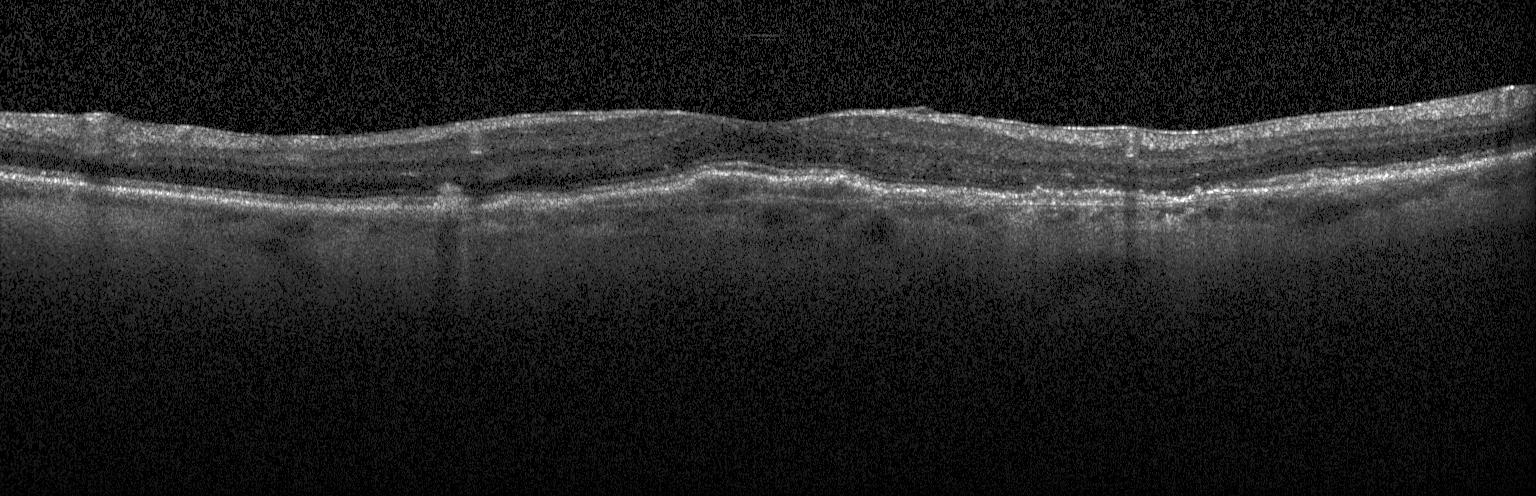

Choroidal neovascularization.